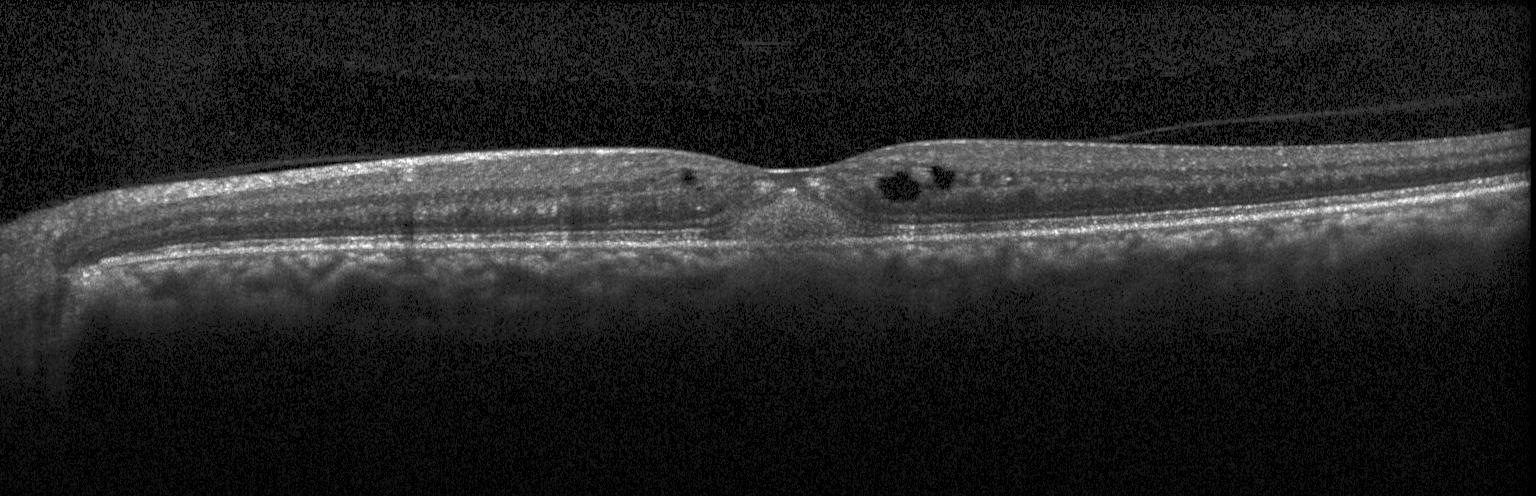

OCT B-scan, through the macula, spectral-domain optical coherence tomography.
Macular OCT: choroidal neovascularization (CNV).